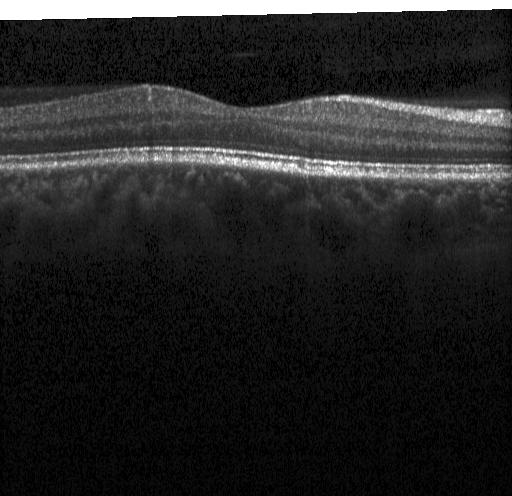
Spectral-domain OCT; fovea-centered; retinal OCT B-scan
Assessment: no evidence of choroidal neovascularization, diabetic macular edema, or drusen.